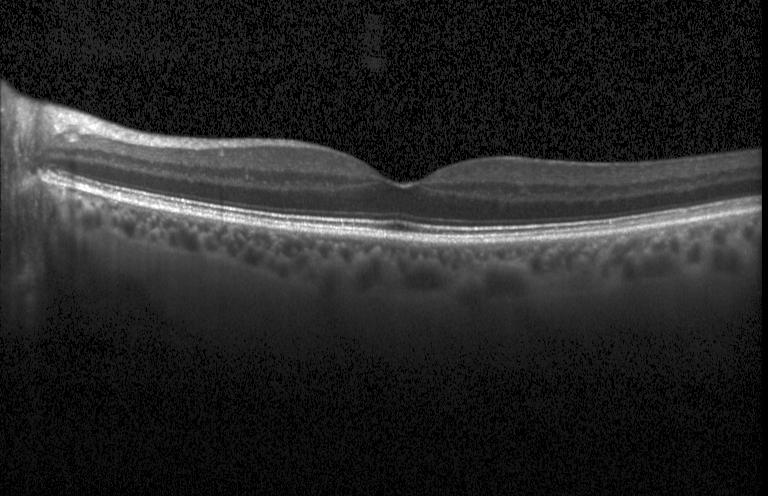

Instrument: Heidelberg Spectralis · spectral-domain OCT · OCT line scan
Diagnosis: no evidence of CNV, DME, or drusen.